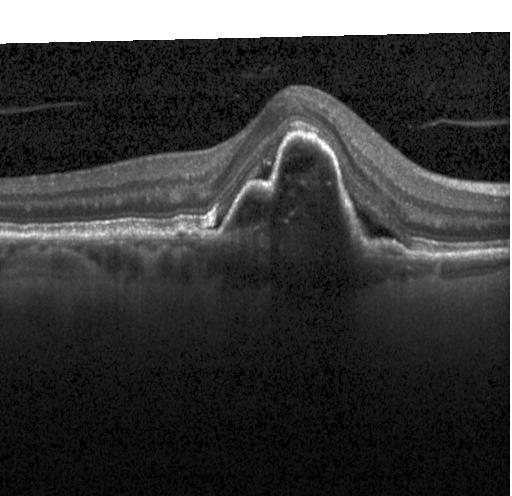

Retinal OCT cross-section; spectral-domain OCT; centered on the fovea; Heidelberg Spectralis OCT system
Finding: a choroidal neovascular membrane.